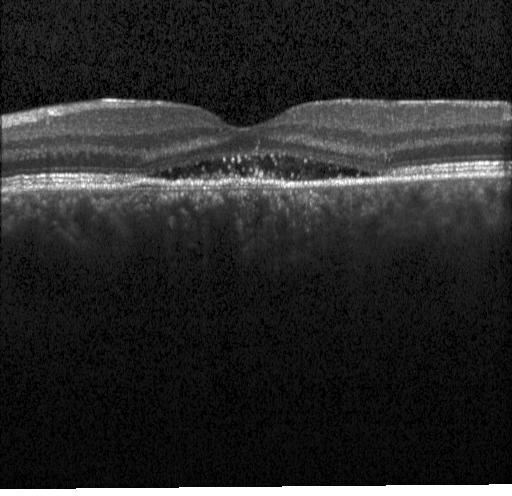

Impression: a choroidal neovascular membrane.